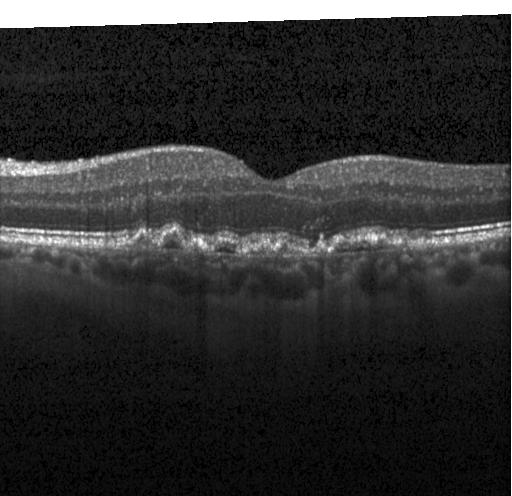
Retinal OCT cross-section — Impression: multiple drusen.